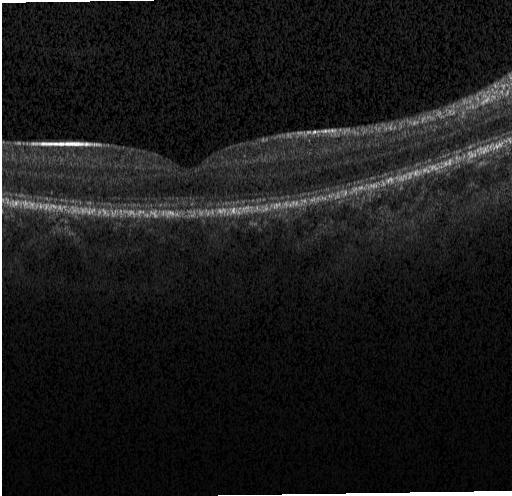
Fovea-centered. Optical coherence tomography B-scan
OCT finding: no evidence of CNV, DME, or drusen.